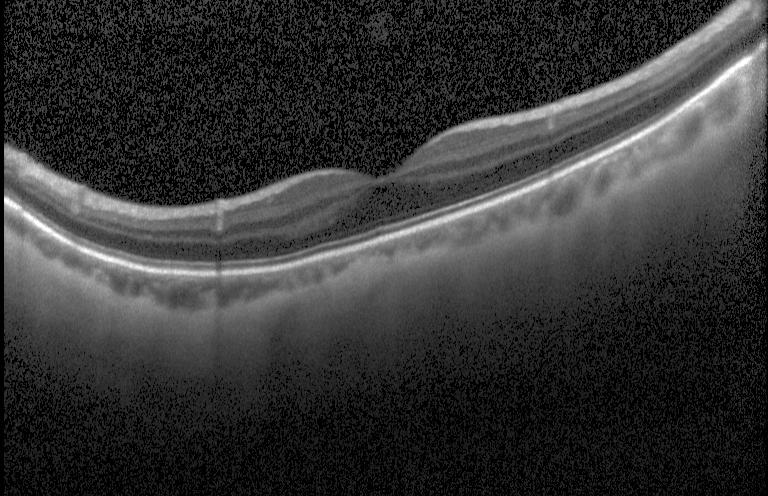

Impression: no choroidal neovascularization, no diabetic macular edema, and no drusen.